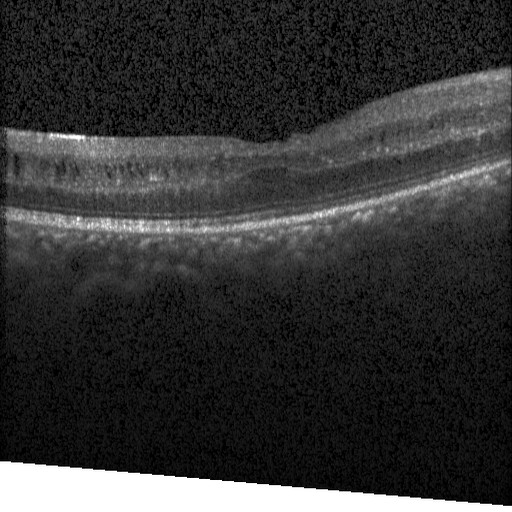

Finding: diabetic macular edema.